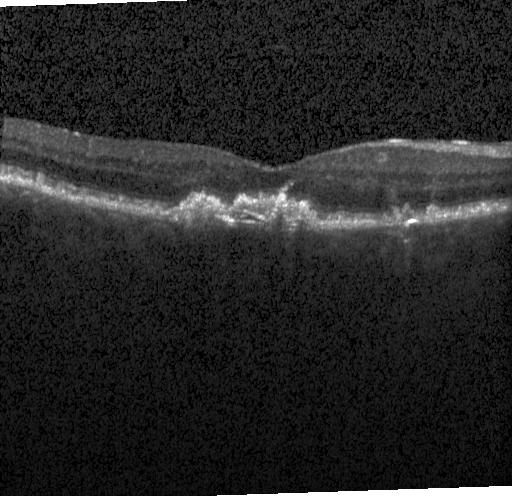 This B-scan demonstrates CNV.